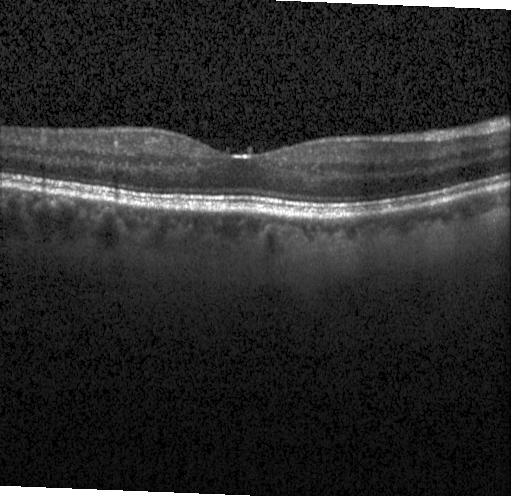 Optical coherence tomography scan. Heidelberg Spectralis OCT system. Macular scan. Dx: neither choroidal neovascularization, diabetic macular edema, nor drusen.